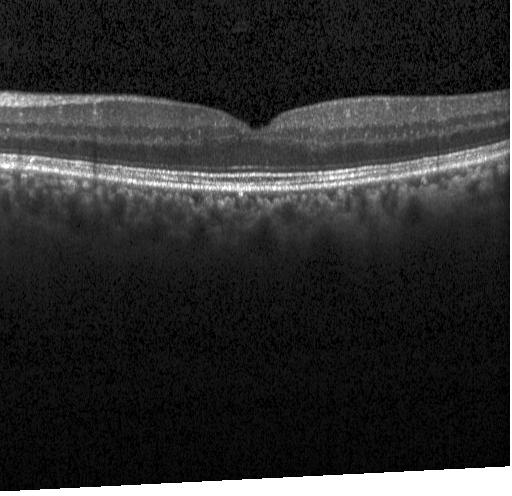

Acquired on a Heidelberg Spectralis; retinal OCT cross-section; macular scan; spectral-domain OCT.
OCT finding: no CNV, no DME, and no drusen.